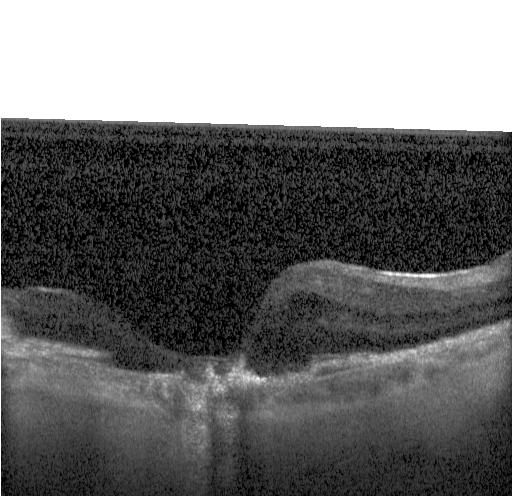 OCT B-scan. SD-OCT. Diagnosis: a choroidal neovascular membrane.